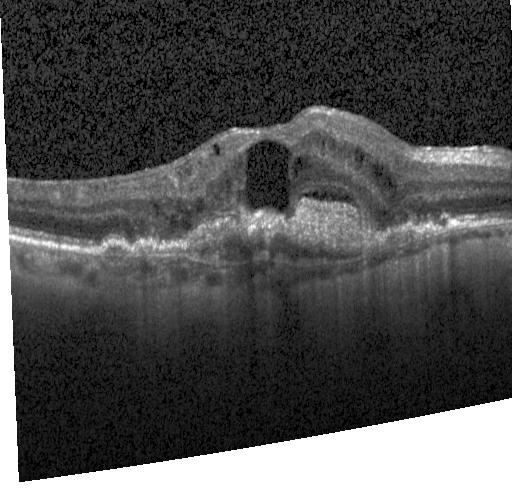 Optical coherence tomography scan · spectral-domain OCT.
Finding: a choroidal neovascular membrane.